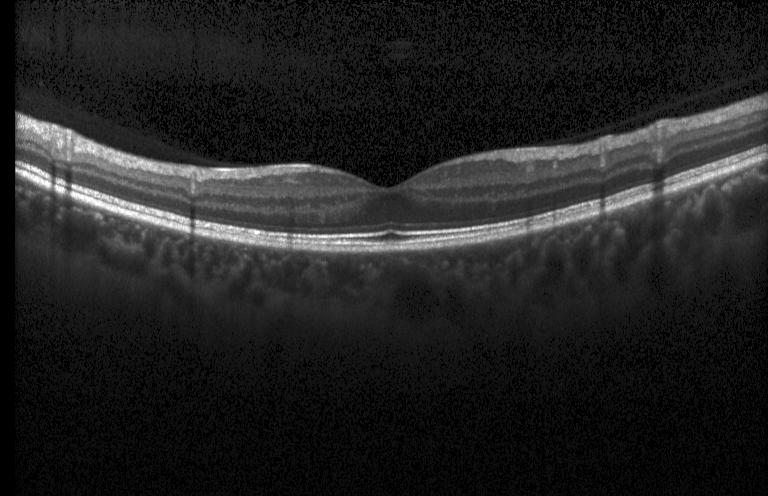 Acquired on a Heidelberg Spectralis; OCT line scan.
Impression: no choroidal neovascularization, diabetic macular edema, or drusen.